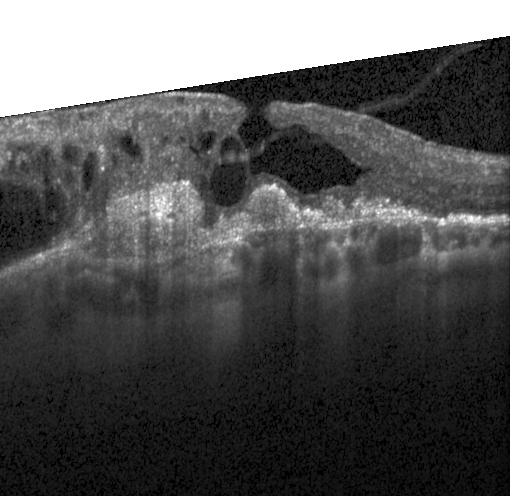

Through the macula. Retinal OCT cross-section. Spectral-domain OCT
Finding: choroidal neovascularization.